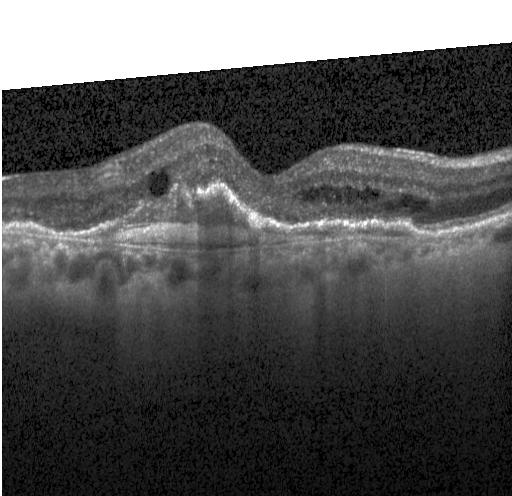

Spectral-domain OCT. Optical coherence tomography B-scan. Instrument: Heidelberg Spectralis. Centered on the fovea — Dx: a choroidal neovascular membrane.